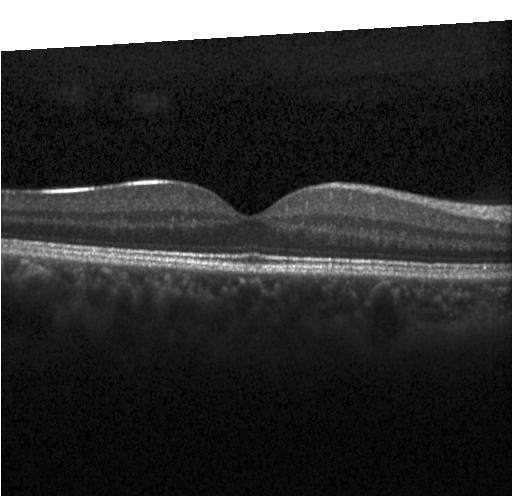 Centered on the fovea · retinal OCT cross-section · SD-OCT — Impression: no evidence of choroidal neovascularization, diabetic macular edema, or drusen.